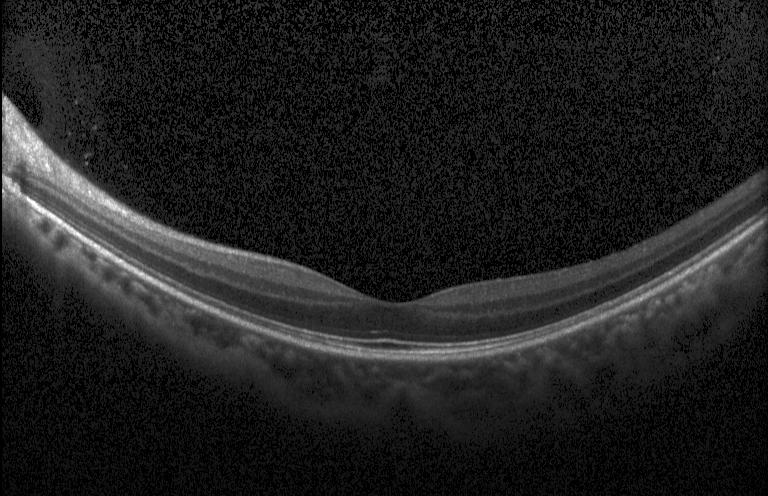
Retinal OCT cross-section.
Finding: neither choroidal neovascularization, diabetic macular edema, nor drusen.